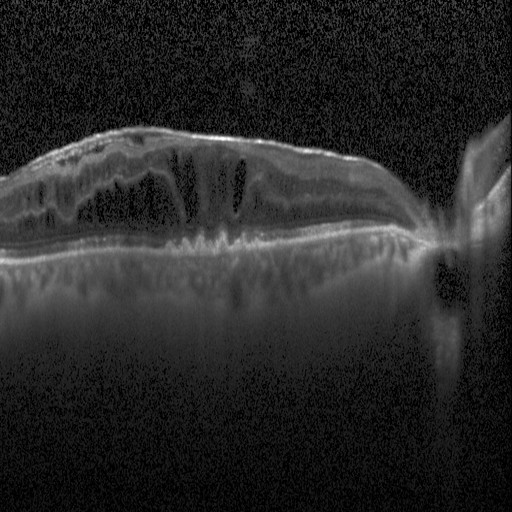 Optical coherence tomography scan
Finding: DME.